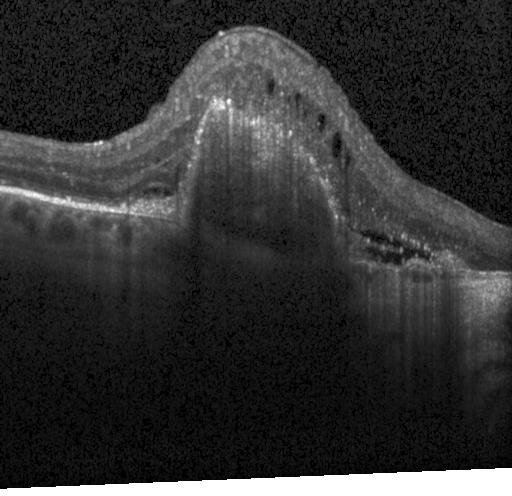
OCT B-scan. Macular OCT: a choroidal neovascular membrane.